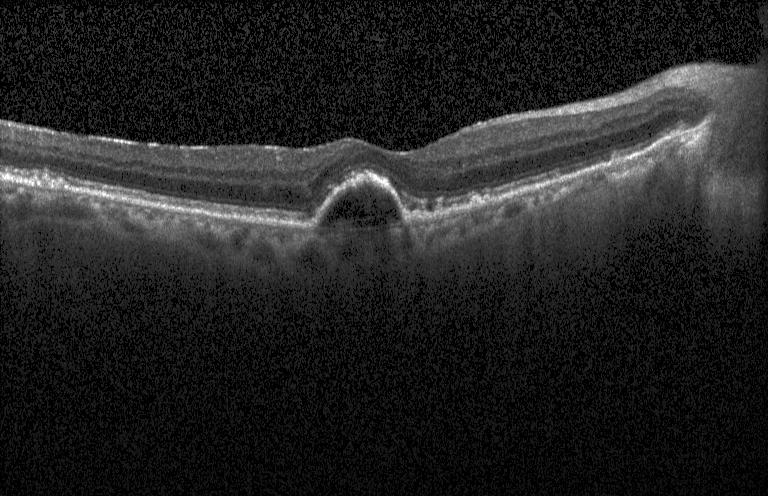 Spectral-domain OCT · retinal OCT B-scan · through the macula.
Dx: a choroidal neovascular membrane.